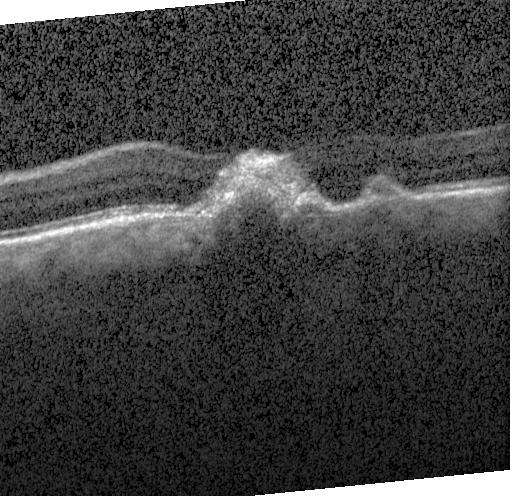

Dx: CNV.